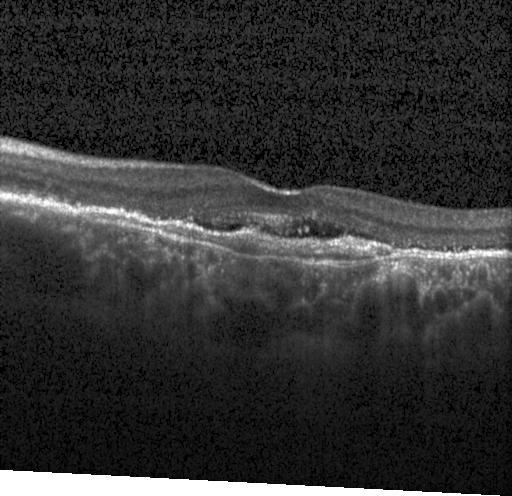 Horizontal scan through the fovea · optical coherence tomography scan. Impression: CNV.